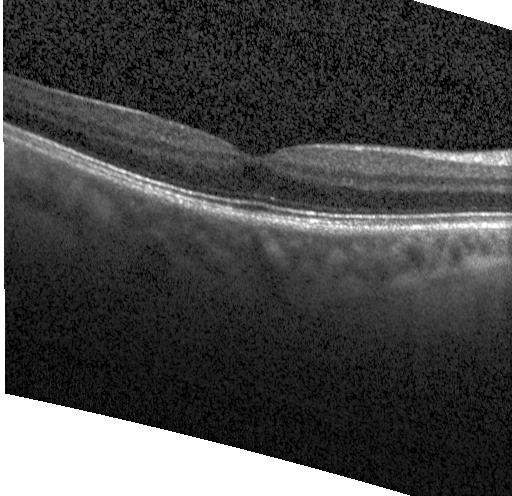
Optical coherence tomography B-scan, Heidelberg Spectralis OCT system
Impression: neither choroidal neovascularization, diabetic macular edema, nor drusen.